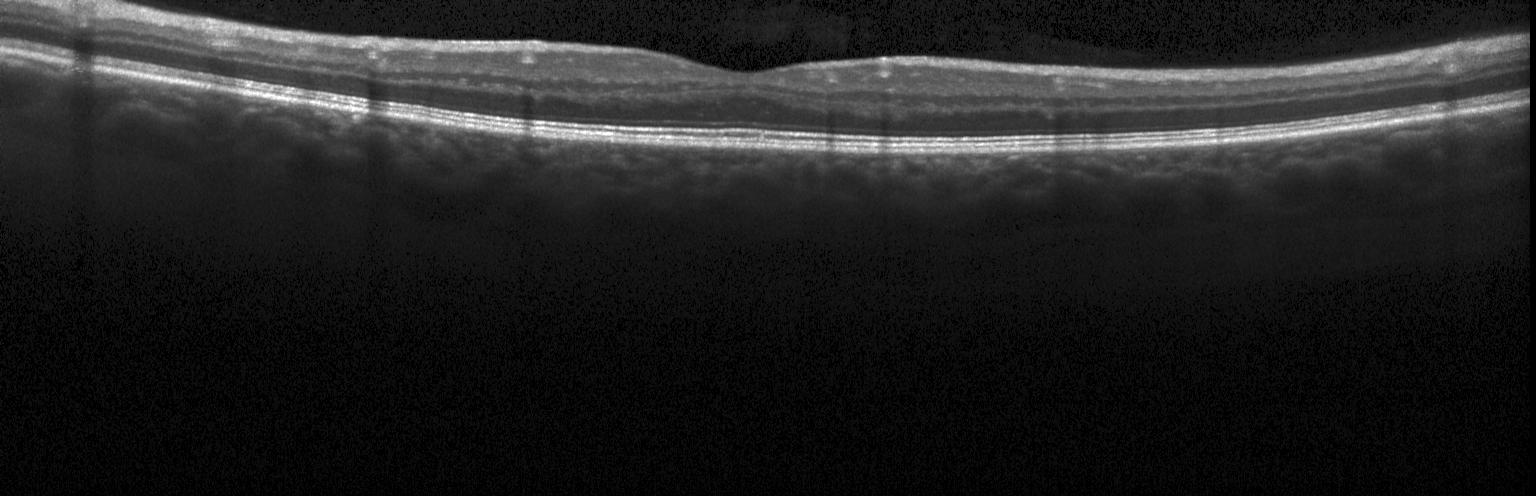 The scan shows no evidence of choroidal neovascularization, diabetic macular edema, or drusen.